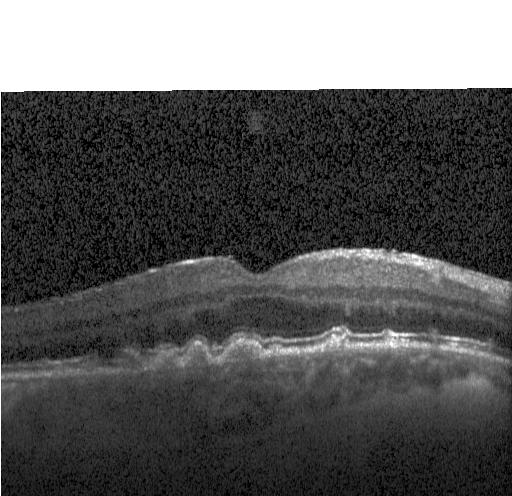
Retinal OCT cross-section. Centered on the fovea. Heidelberg Spectralis OCT system. SD-OCT — Assessment: drusen.